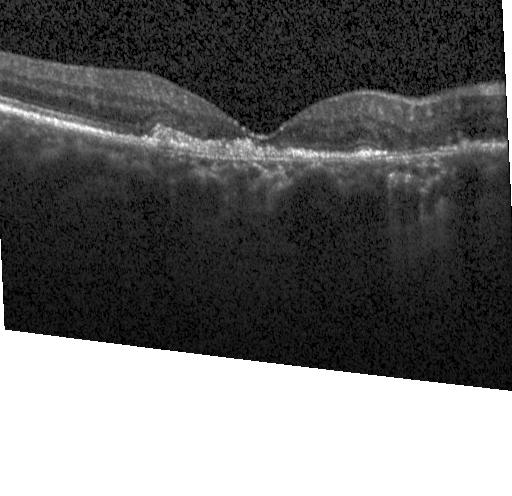

Spectral-domain OCT; centered on the fovea; optical coherence tomography scan.
Choroidal neovascularization (CNV).